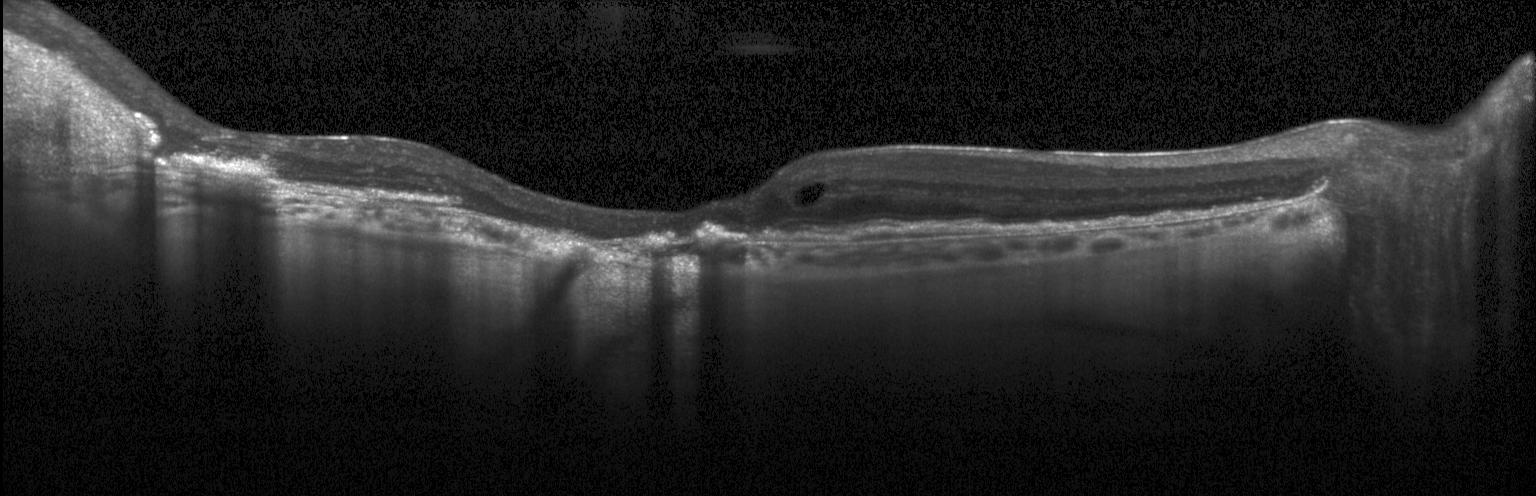

Spectral-domain optical coherence tomography, horizontal scan through the fovea, optical coherence tomography B-scan, Heidelberg Spectralis
Assessment: a choroidal neovascular membrane.